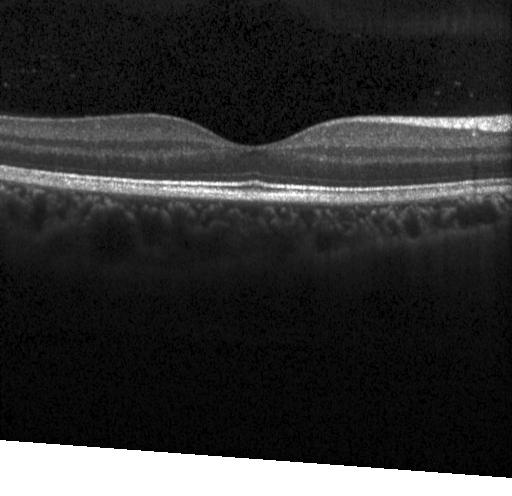
Dx: no choroidal neovascularization, no diabetic macular edema, and no drusen.